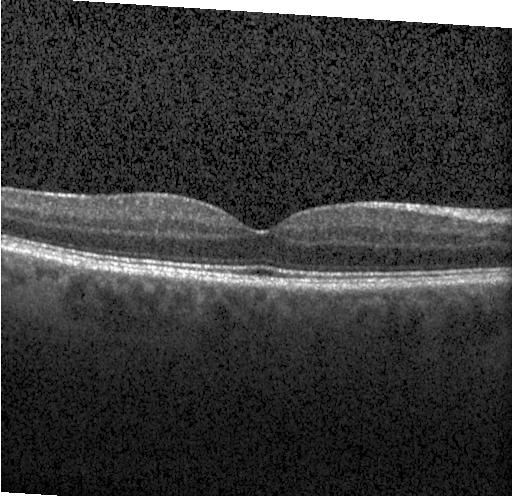
Optical coherence tomography B-scan. SD-OCT.
Diagnosis: no choroidal neovascularization, diabetic macular edema, or drusen.